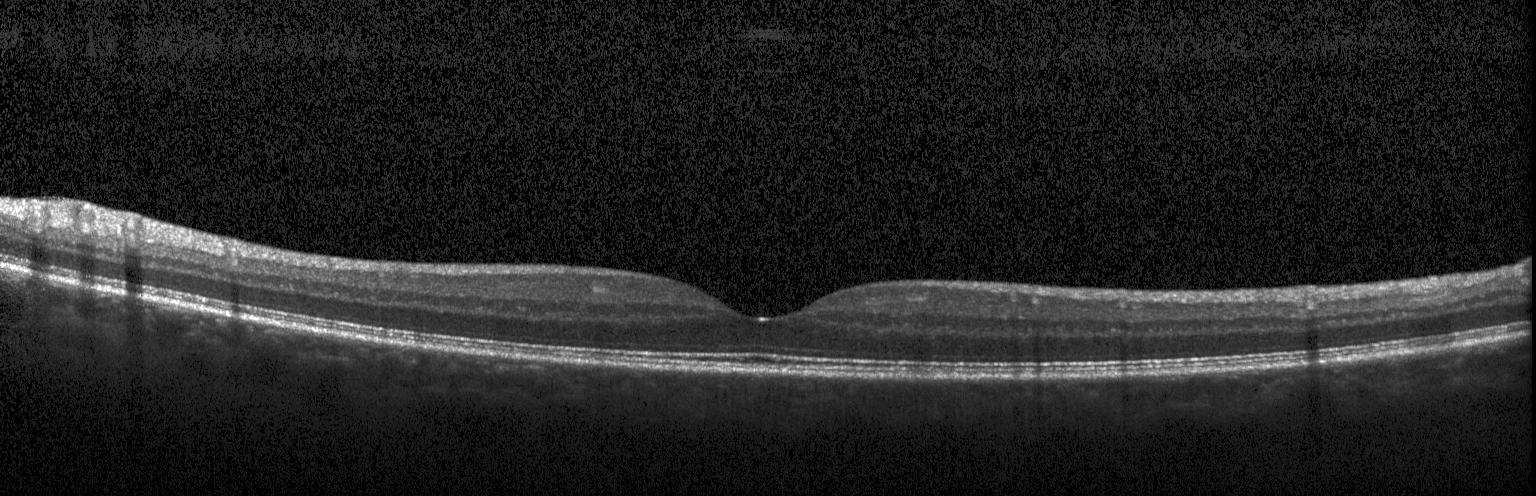

Macular OCT: no CNV, no DME, and no drusen.